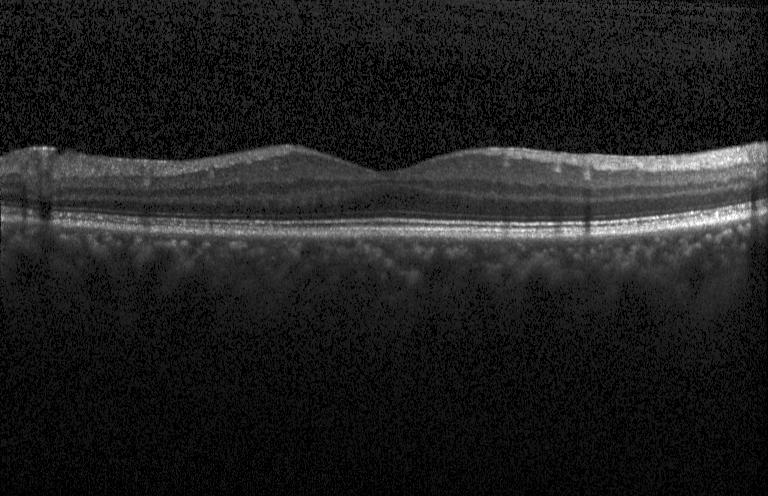 Assessment: no evidence of choroidal neovascularization, diabetic macular edema, or drusen.